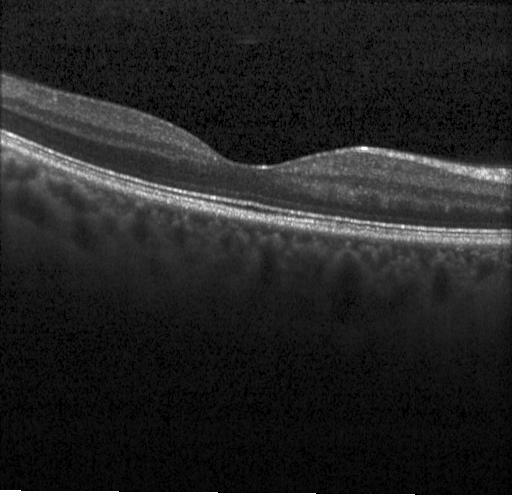

OCT line scan
Impression: neither choroidal neovascularization, diabetic macular edema, nor drusen.